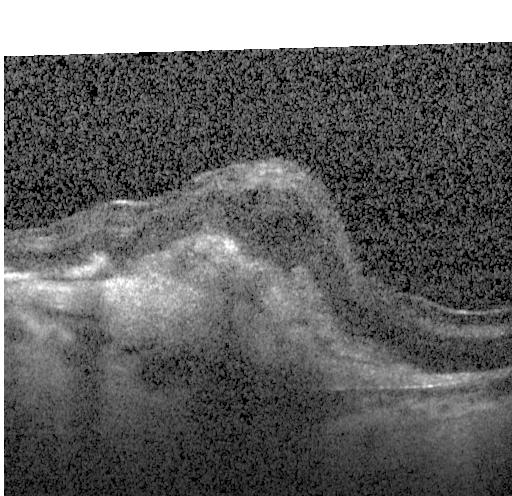 Spectral-domain optical coherence tomography. Instrument: Heidelberg Spectralis. OCT B-scan. Fovea-centered.
Choroidal neovascularization (CNV).